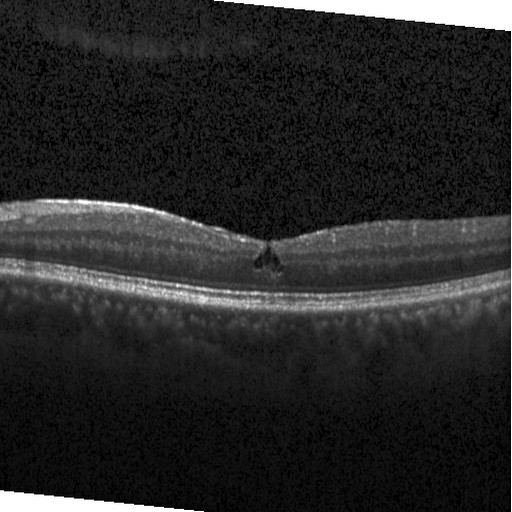
Heidelberg Spectralis · retinal OCT cross-section · SD-OCT · through the macula
Assessment: diabetic macular edema.